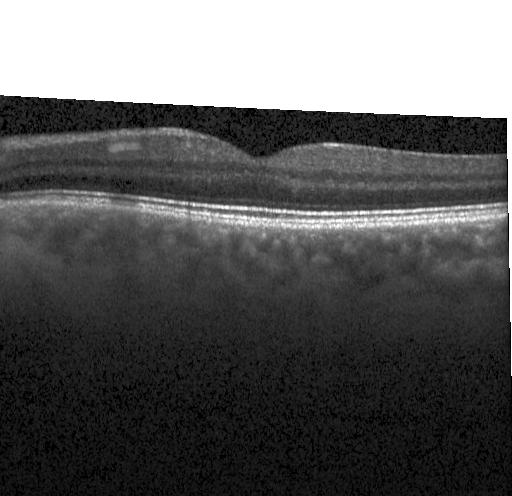 The scan shows no choroidal neovascularization, diabetic macular edema, or drusen.